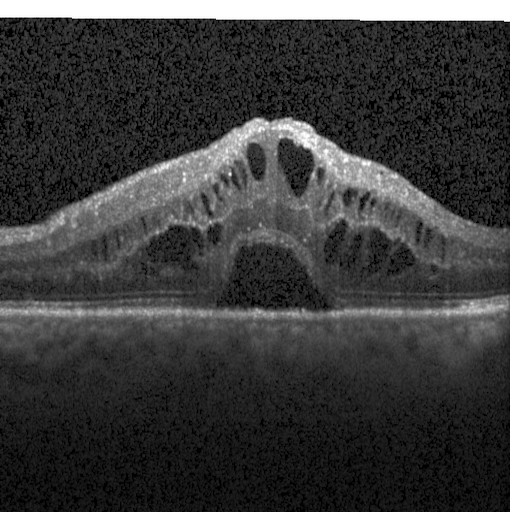 Centered on the fovea. OCT B-scan. Heidelberg Spectralis. This B-scan demonstrates diabetic macular edema.